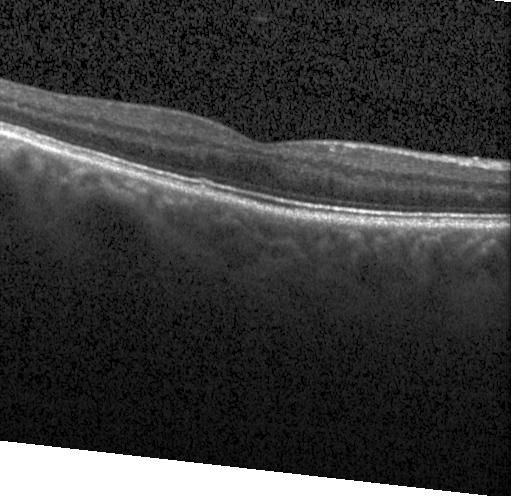

Spectral-domain optical coherence tomography; OCT line scan; horizontal scan through the fovea; acquired on a Heidelberg Spectralis.
Impression: no evidence of choroidal neovascularization, diabetic macular edema, or drusen.